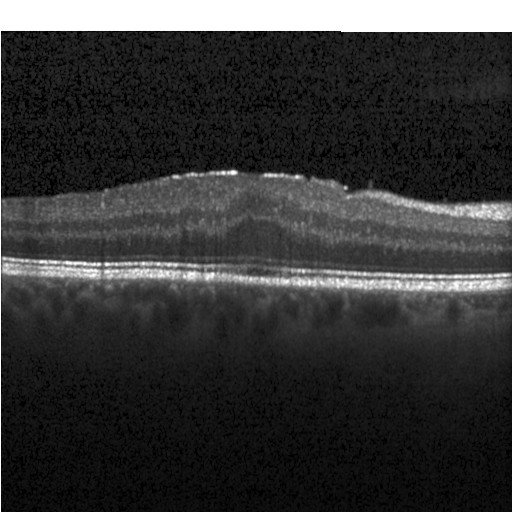

Finding: diabetic macular edema.